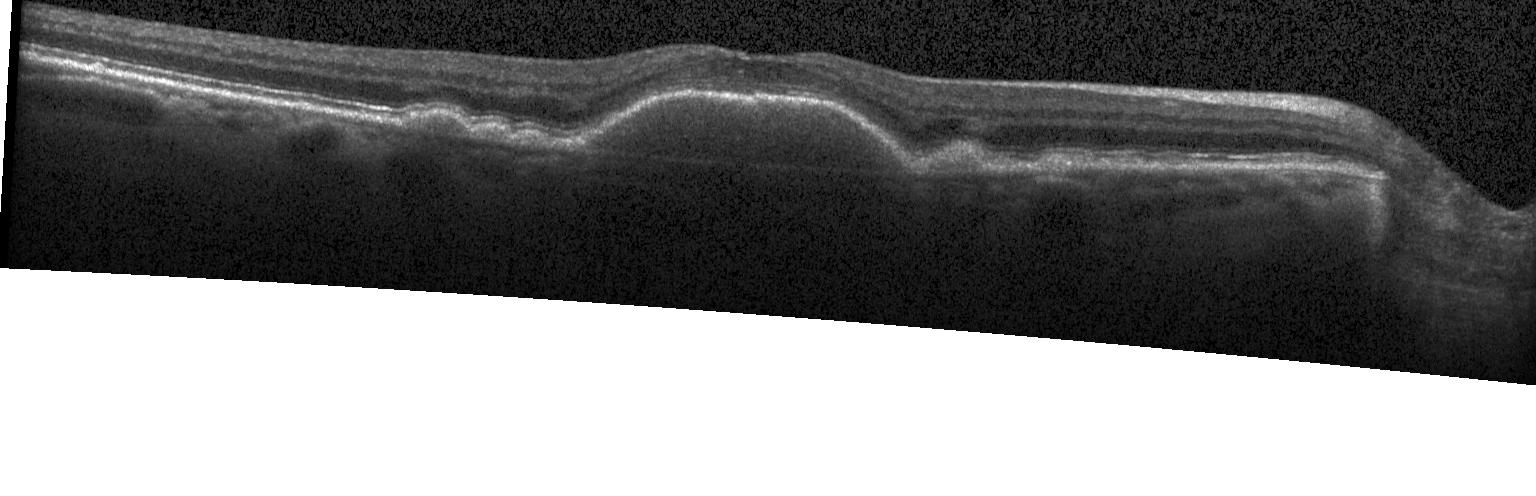 OCT B-scan
Diagnosis: a choroidal neovascular membrane.